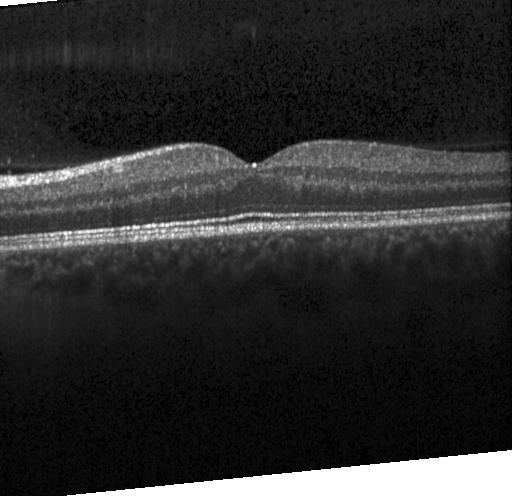
SD-OCT, horizontal scan through the fovea, acquired on a Heidelberg Spectralis, OCT B-scan — Diagnosis: no choroidal neovascularization, diabetic macular edema, or drusen.